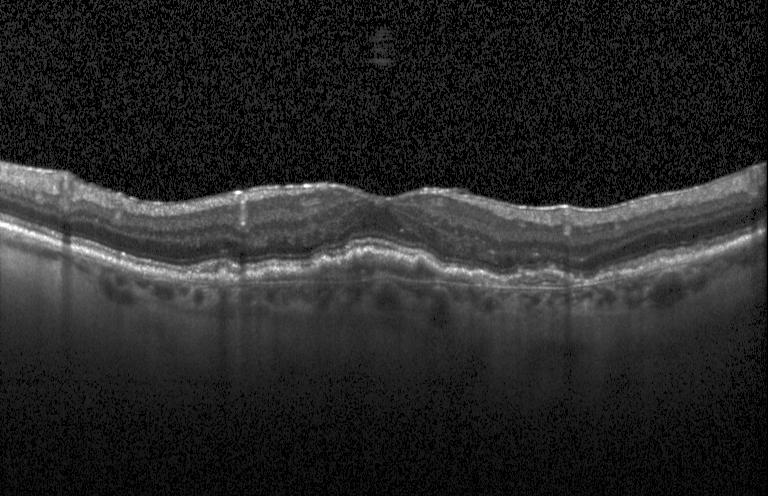
OCT B-scan. Macular scan — Diagnosis: choroidal neovascularization.